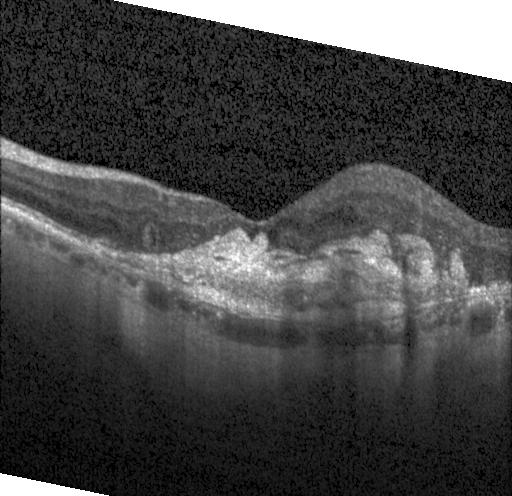
Assessment: a choroidal neovascular membrane.